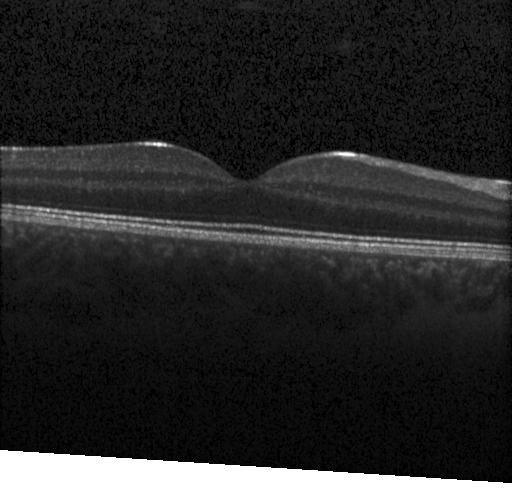
Heidelberg Spectralis; optical coherence tomography scan; spectral-domain OCT
Macular OCT: neither CNV, DME, nor drusen.